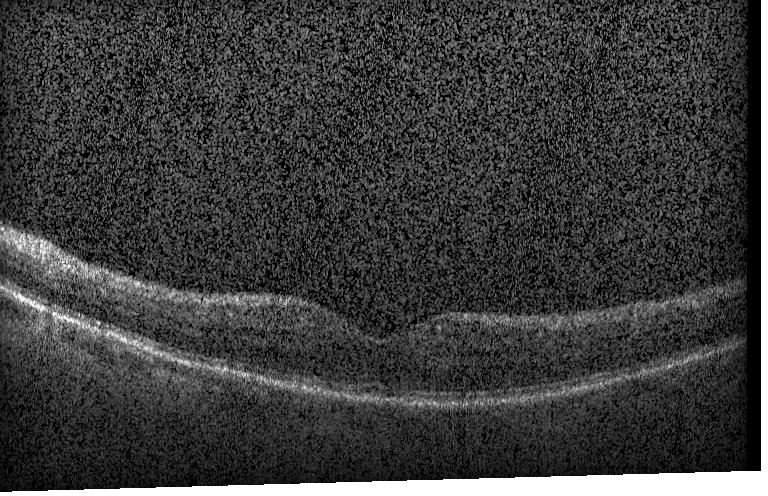 Instrument: Heidelberg Spectralis. Retinal OCT B-scan. Macular scan. Spectral-domain OCT
Impression: no choroidal neovascularization, diabetic macular edema, or drusen.